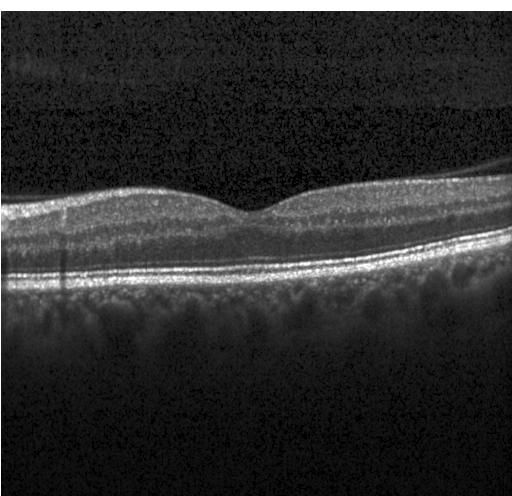
Retinal OCT cross-section showing no CNV, DME, or drusen.